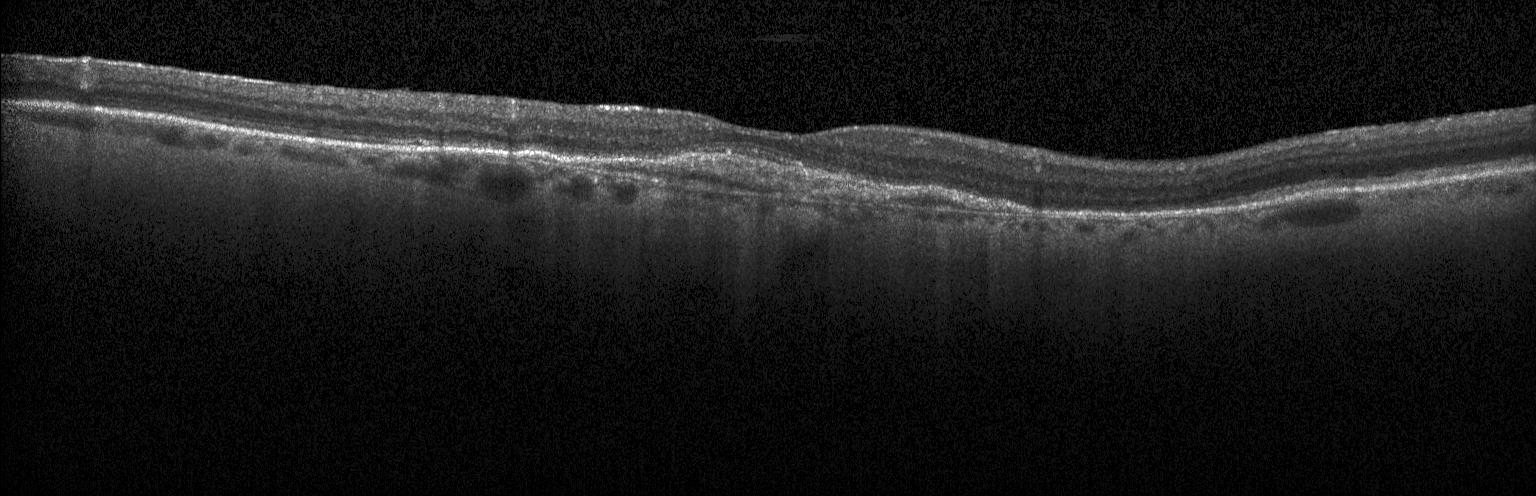
Spectral-domain optical coherence tomography; optical coherence tomography B-scan; instrument: Heidelberg Spectralis.
OCT finding: a choroidal neovascular membrane.